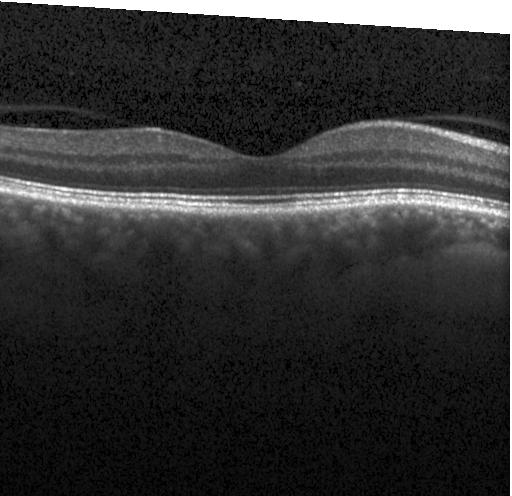
OCT B-scan; spectral-domain optical coherence tomography; Heidelberg Spectralis
The scan shows no choroidal neovascularization, diabetic macular edema, or drusen.